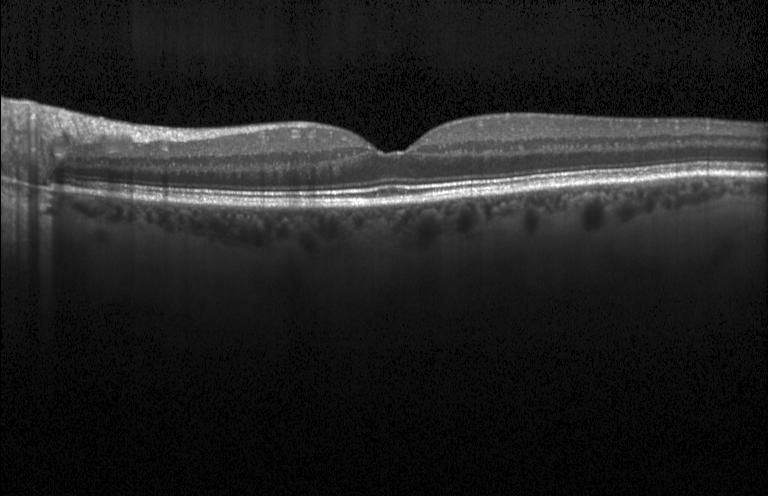 OCT B-scan · Heidelberg Spectralis OCT system · SD-OCT
This B-scan demonstrates no choroidal neovascularization, no diabetic macular edema, and no drusen.